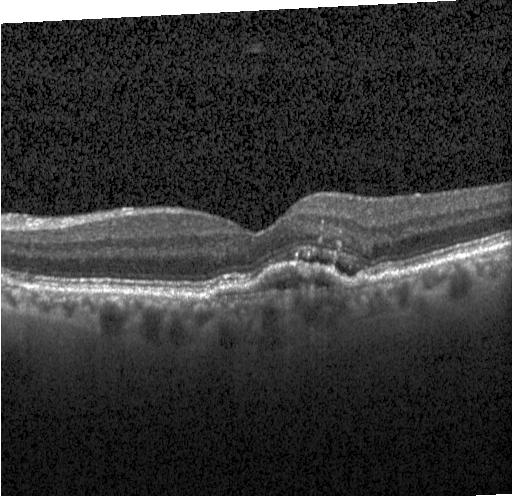 Heidelberg Spectralis OCT system · retinal OCT B-scan · spectral-domain optical coherence tomography · through the macula.
Finding: a choroidal neovascular membrane.